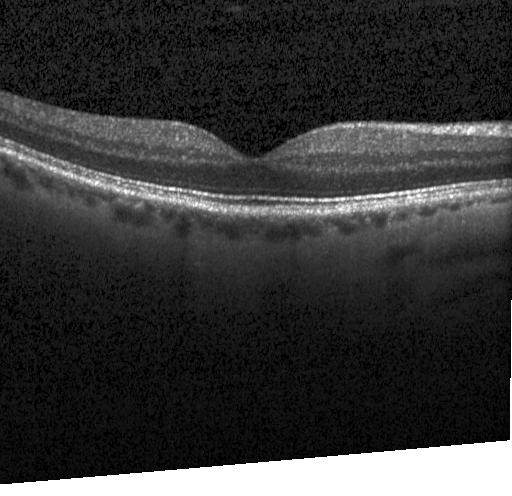
Optical coherence tomography scan · Heidelberg Spectralis · horizontal scan through the fovea
This B-scan demonstrates neither choroidal neovascularization, diabetic macular edema, nor drusen.